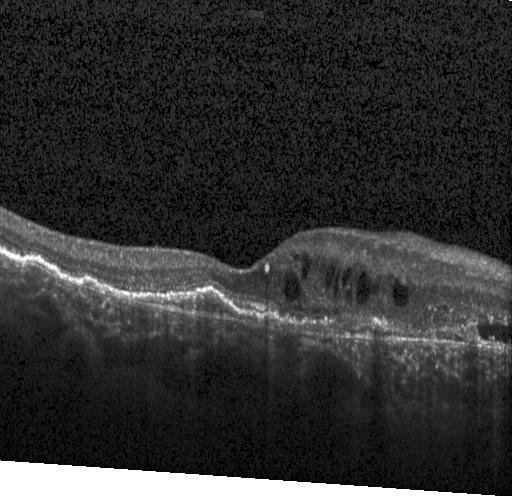
Finding: a choroidal neovascular membrane.